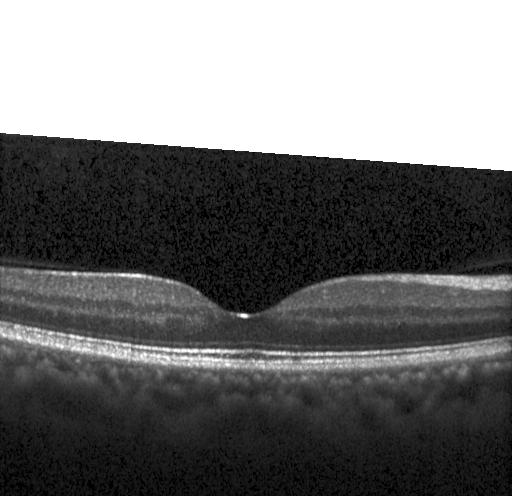 Spectral-domain optical coherence tomography · optical coherence tomography B-scan — Impression: no evidence of choroidal neovascularization, diabetic macular edema, or drusen.